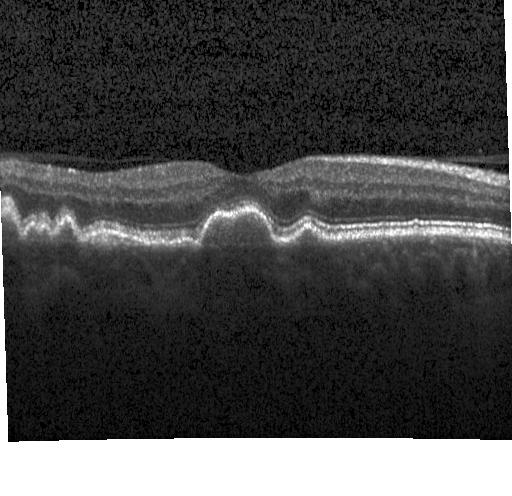 SD-OCT · retinal OCT B-scan
Sub-RPE drusenoid deposits.